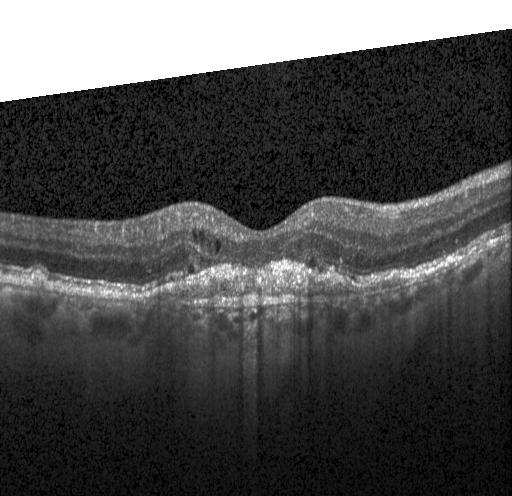 Retinal OCT cross-section
A choroidal neovascular membrane.